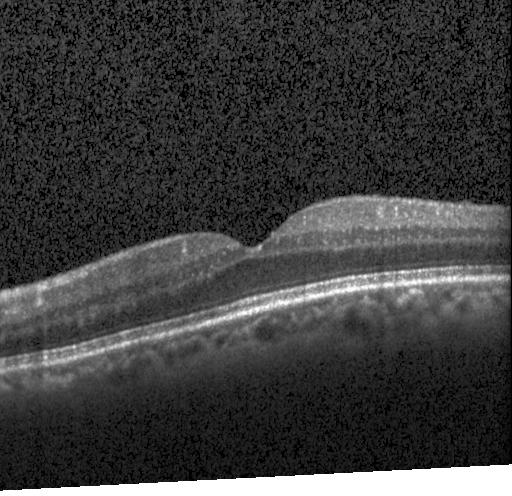

Optical coherence tomography B-scan. Heidelberg Spectralis — Macular OCT: no evidence of choroidal neovascularization, diabetic macular edema, or drusen.